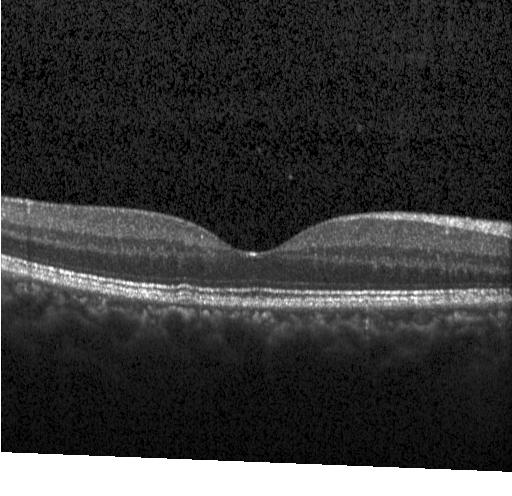
Optical coherence tomography scan.
OCT finding: drusen.